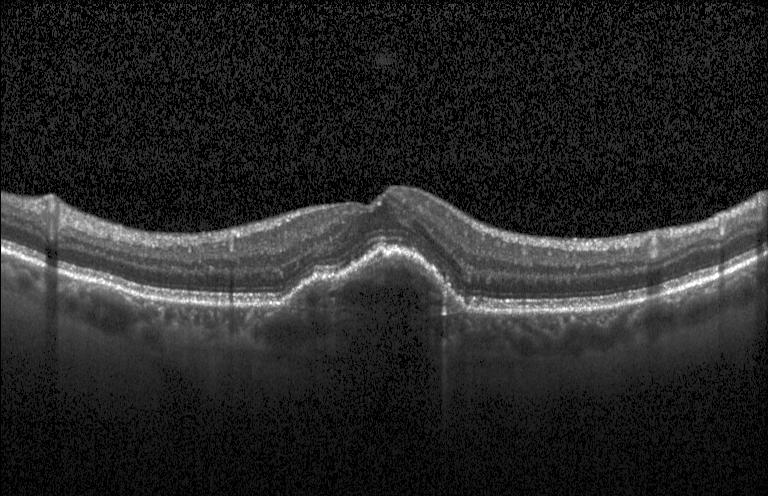 Fovea-centered · spectral-domain optical coherence tomography · OCT line scan — Assessment: choroidal neovascularization (CNV).